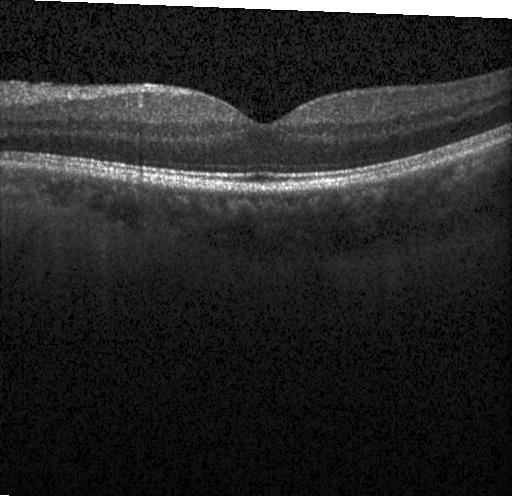 OCT B-scan.
Finding: no choroidal neovascularization, no diabetic macular edema, and no drusen.